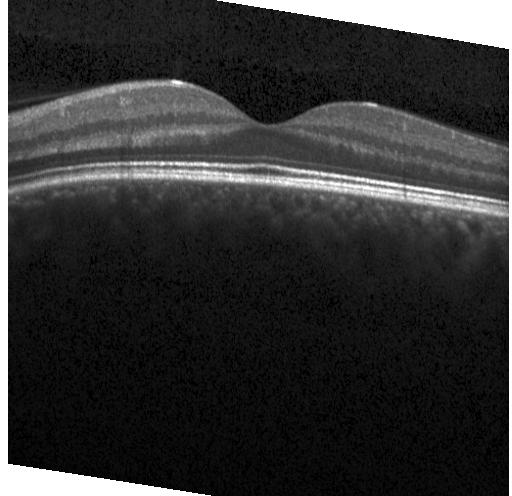 Retinal OCT B-scan, spectral-domain OCT.
Finding: neither choroidal neovascularization, diabetic macular edema, nor drusen.